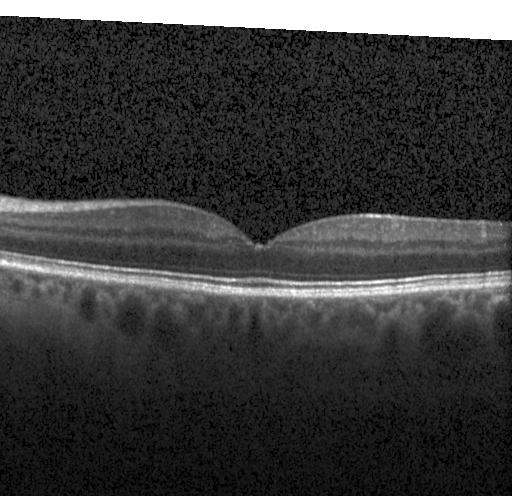
OCT B-scan showing no CNV, DME, or drusen.